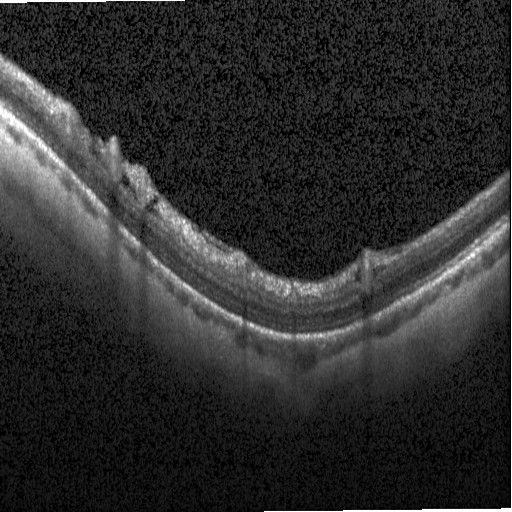

Horizontal scan through the fovea. Spectral-domain optical coherence tomography. OCT B-scan. Heidelberg Spectralis OCT system
Dx: diabetic macular edema.